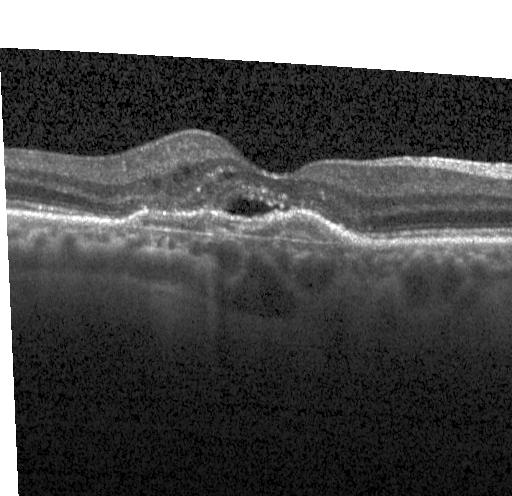 Retinal OCT cross-section. Instrument: Heidelberg Spectralis. Spectral-domain optical coherence tomography. Through the macula. The scan shows CNV.